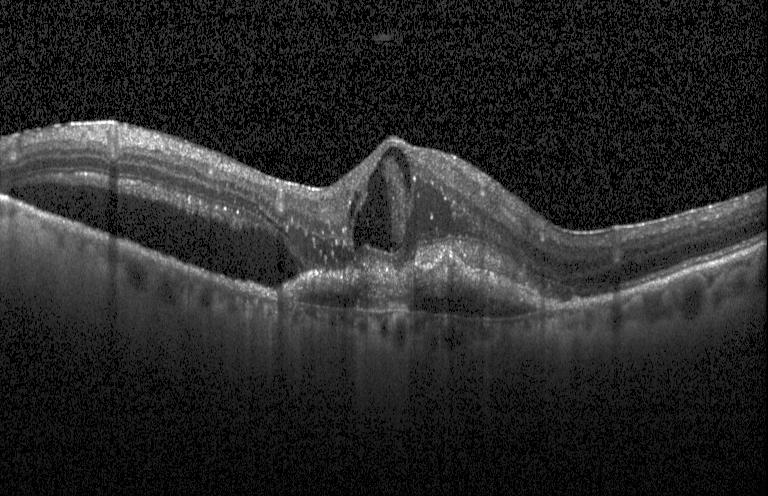
Spectral-domain OCT B-scan: a choroidal neovascular membrane.